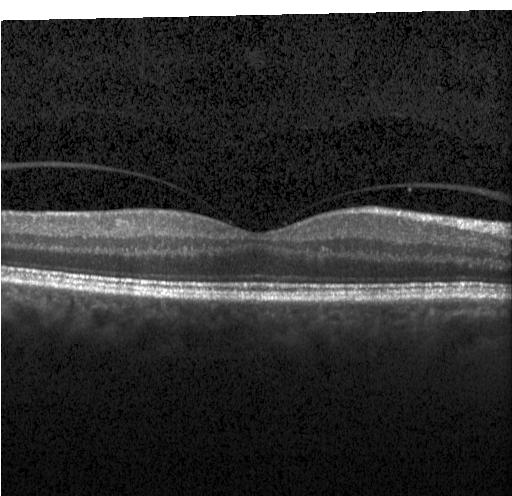
Spectral-domain OCT; OCT line scan — The scan shows no choroidal neovascularization, no diabetic macular edema, and no drusen.